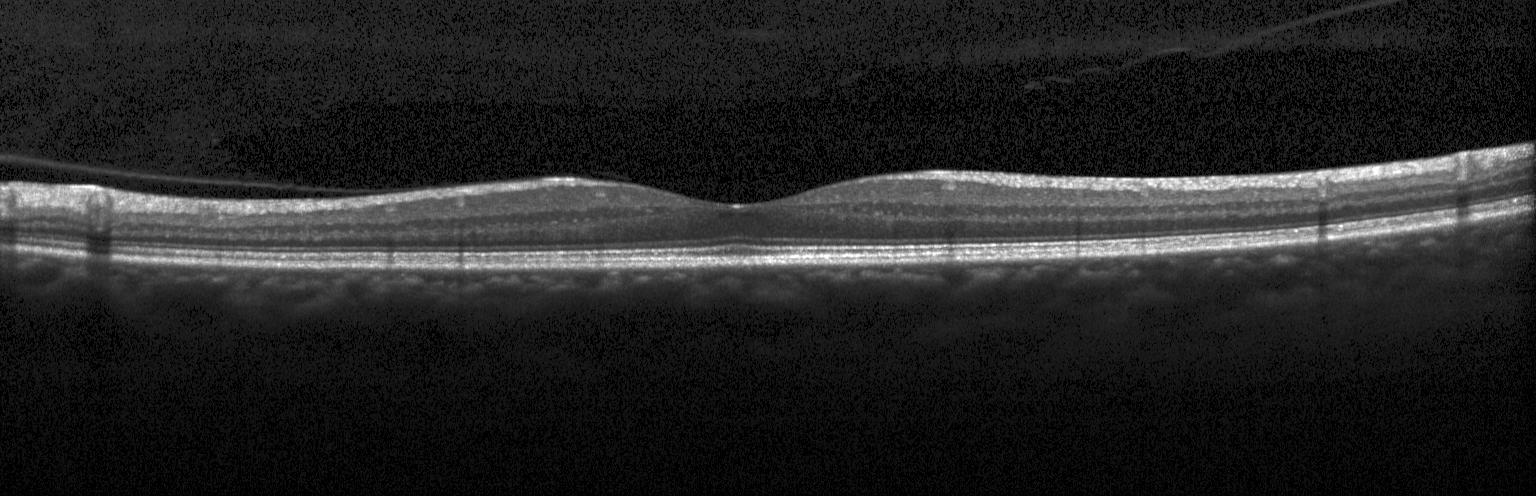

Instrument: Heidelberg Spectralis; SD-OCT; horizontal scan through the fovea; retinal OCT B-scan — Impression: no choroidal neovascularization, no diabetic macular edema, and no drusen.